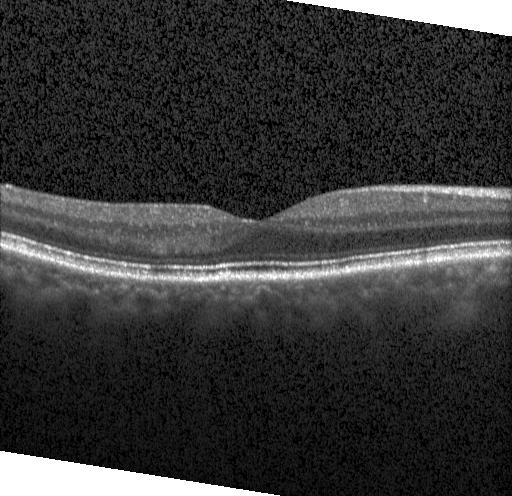

Diagnosis: no CNV, DME, or drusen.